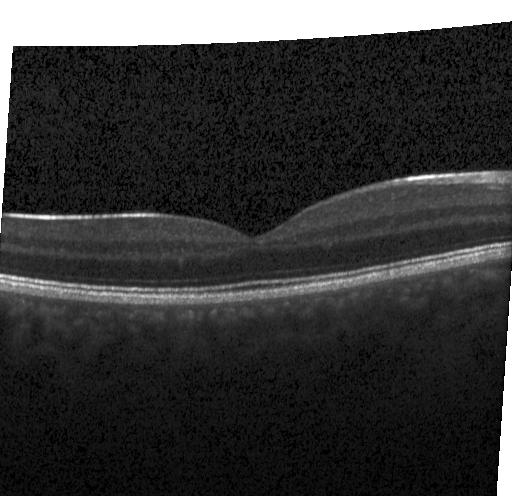

Centered on the fovea, spectral-domain optical coherence tomography, optical coherence tomography B-scan. Dx: no evidence of choroidal neovascularization, diabetic macular edema, or drusen.